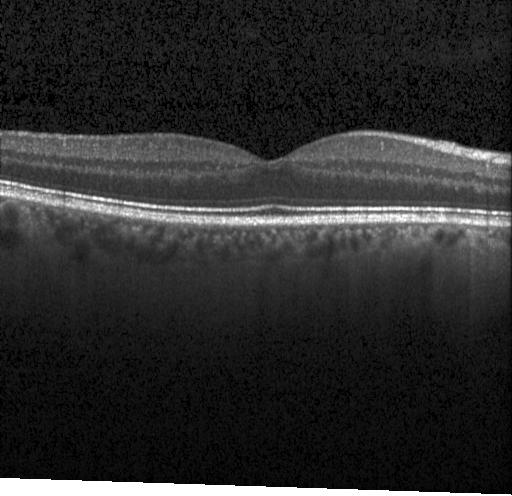 Retinal OCT B-scan; Heidelberg Spectralis.
This B-scan demonstrates no CNV, no DME, and no drusen.